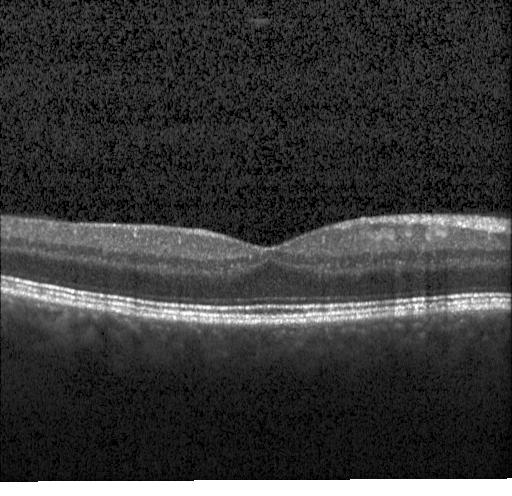
Acquired on a Heidelberg Spectralis, OCT B-scan
Diagnosis: no CNV, DME, or drusen.